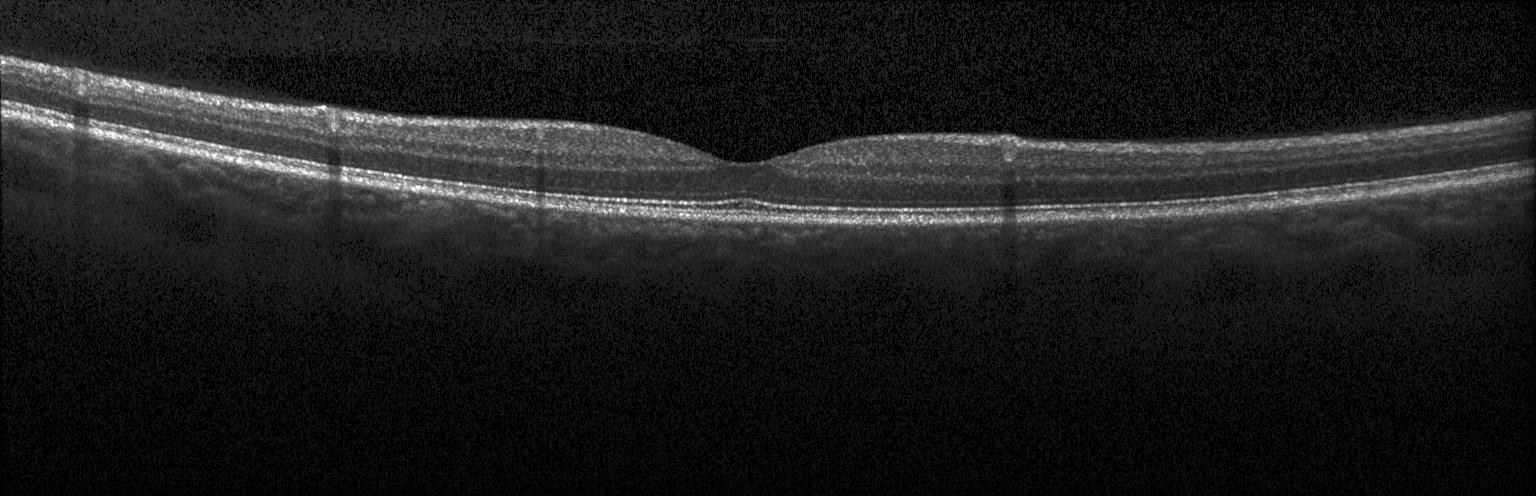 Instrument: Heidelberg Spectralis, horizontal scan through the fovea, optical coherence tomography B-scan, spectral-domain OCT.
The scan shows no evidence of CNV, DME, or drusen.